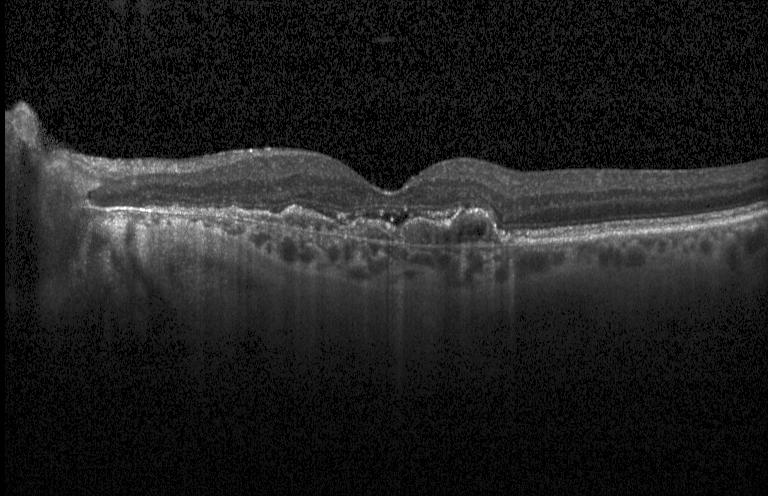
Spectral-domain optical coherence tomography; OCT line scan; instrument: Heidelberg Spectralis; macular scan — Macular OCT: choroidal neovascularization.